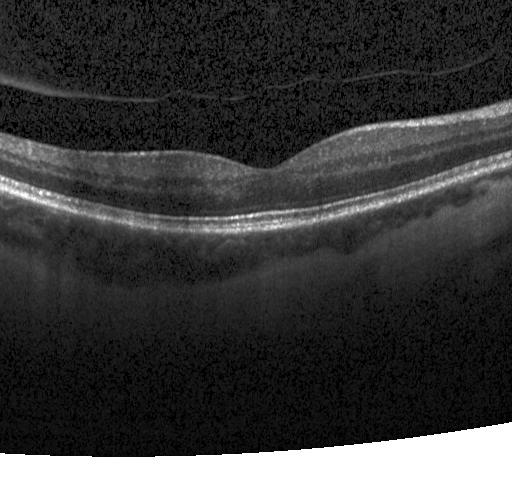
Horizontal scan through the fovea; spectral-domain optical coherence tomography; instrument: Heidelberg Spectralis; retinal OCT cross-section — Impression: no choroidal neovascularization, no diabetic macular edema, and no drusen.